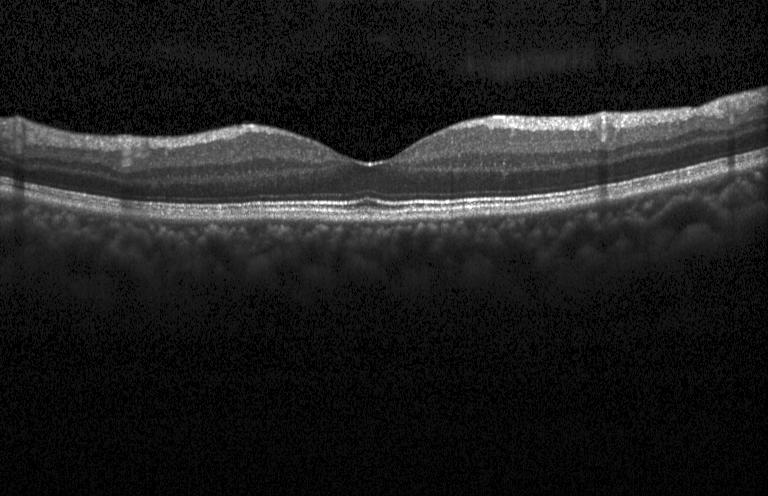
OCT finding: neither choroidal neovascularization, diabetic macular edema, nor drusen.